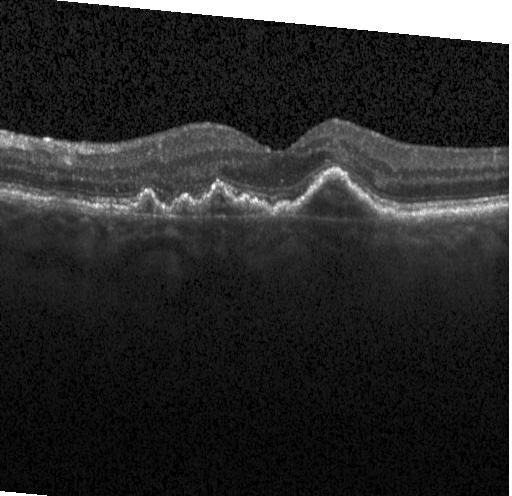
Optical coherence tomography B-scan. SD-OCT. Heidelberg Spectralis OCT system.
Macular OCT: a choroidal neovascular membrane.